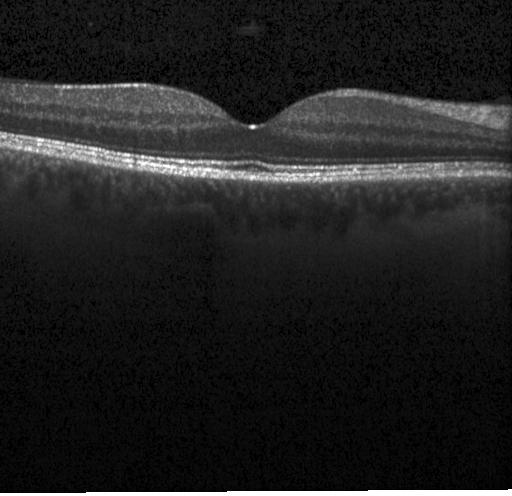 Optical coherence tomography B-scan. Impression: neither CNV, DME, nor drusen.